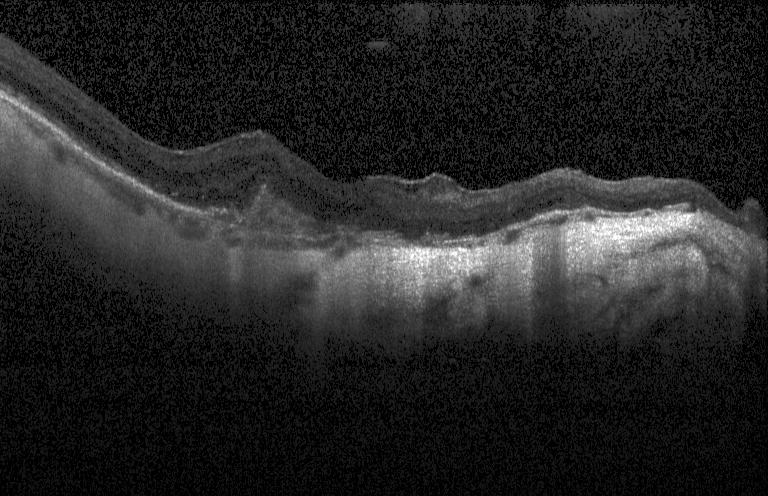

Centered on the fovea, retinal OCT cross-section — Diagnosis: a choroidal neovascular membrane.